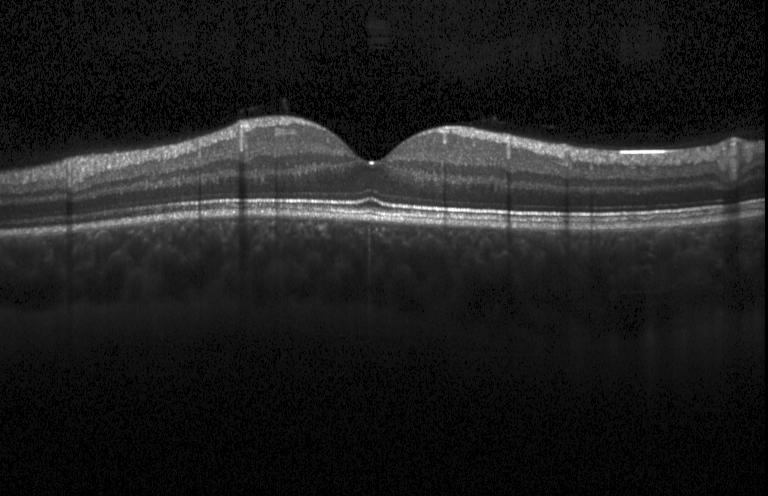 Diagnosis: no CNV, no DME, and no drusen.